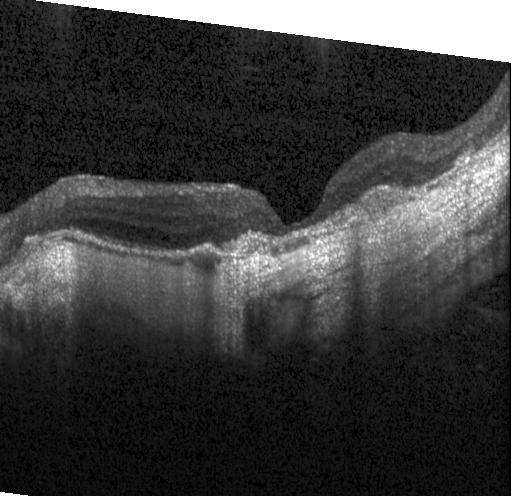 OCT B-scan; macular scan; instrument: Heidelberg Spectralis; spectral-domain optical coherence tomography. Impression: choroidal neovascularization.